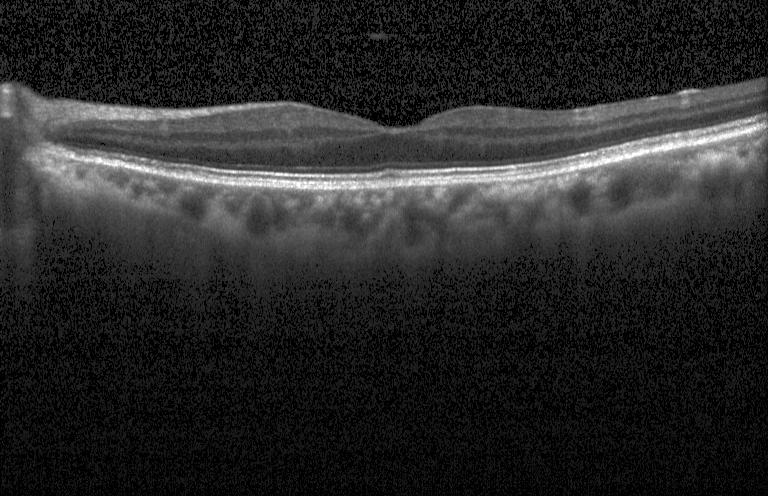
Through the macula, OCT line scan, instrument: Heidelberg Spectralis.
Diagnosis: neither choroidal neovascularization, diabetic macular edema, nor drusen.